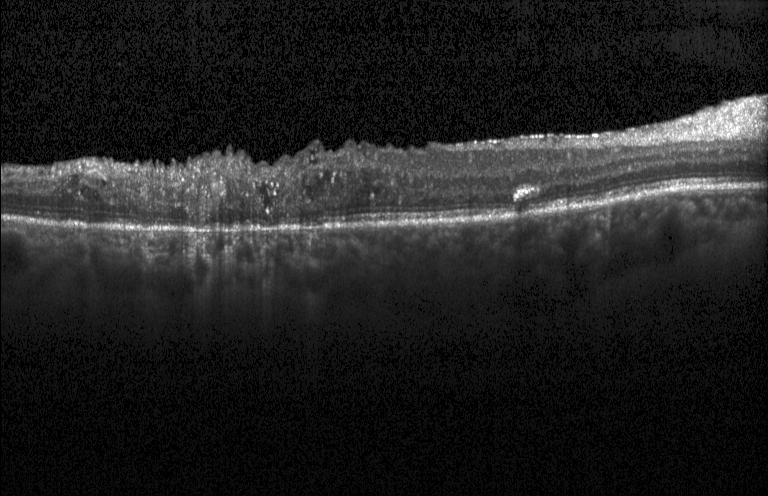 OCT B-scan
Diagnosis: DME.